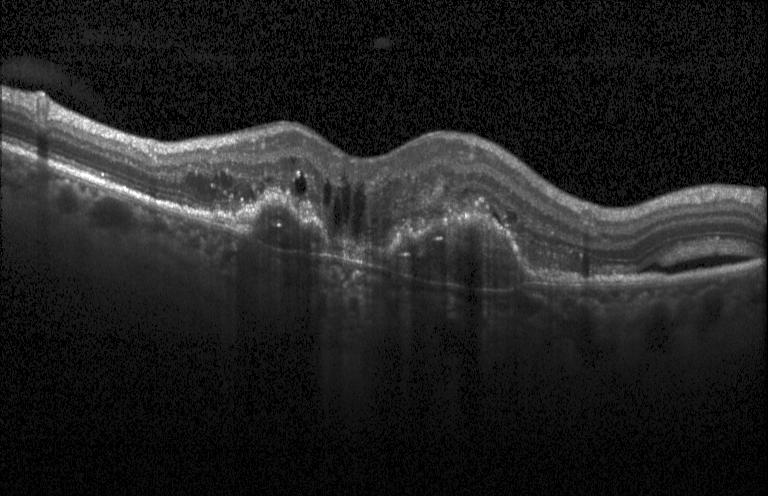

Heidelberg Spectralis OCT system, OCT B-scan. Diagnosis: choroidal neovascularization.